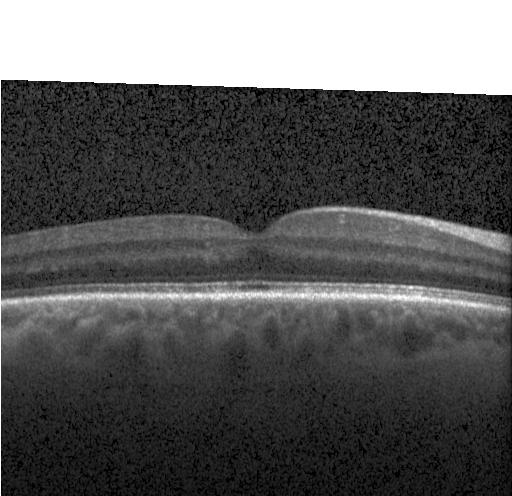
Spectral-domain optical coherence tomography · optical coherence tomography B-scan · Heidelberg Spectralis OCT system
The scan shows no CNV, no DME, and no drusen.